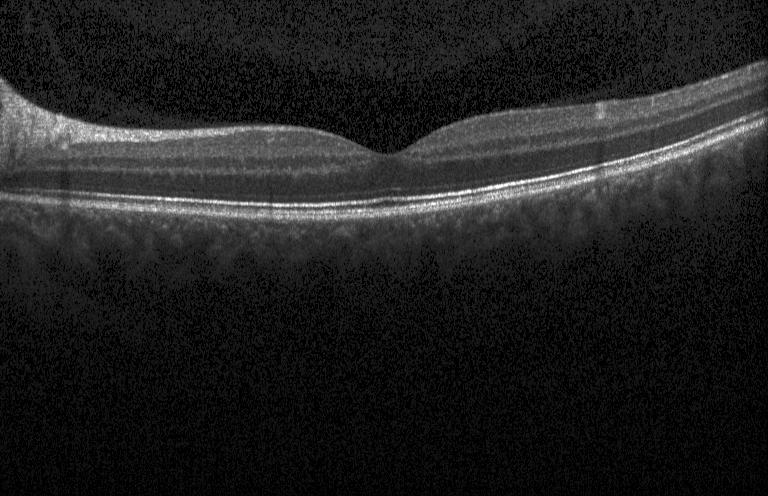

Retinal OCT cross-section. Heidelberg Spectralis OCT system
This B-scan demonstrates no choroidal neovascularization, diabetic macular edema, or drusen.